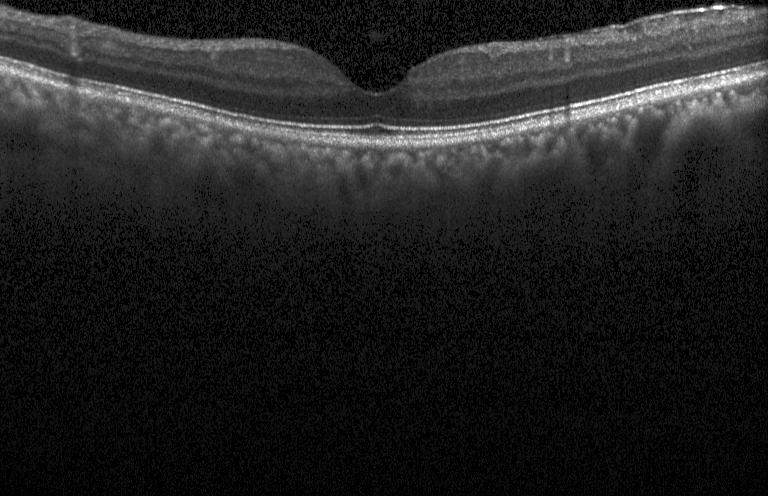
Macular OCT: no CNV, no DME, and no drusen.